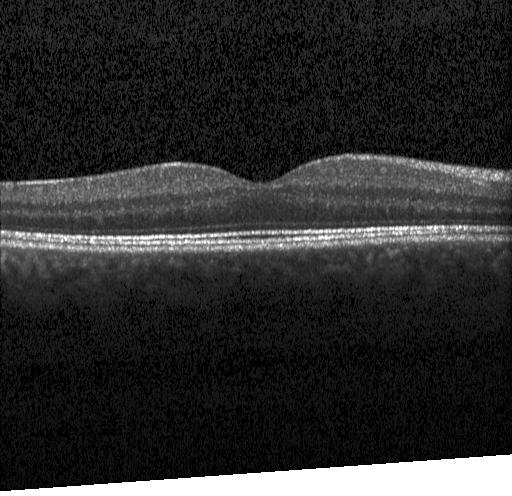

OCT line scan
Assessment: no choroidal neovascularization, diabetic macular edema, or drusen.